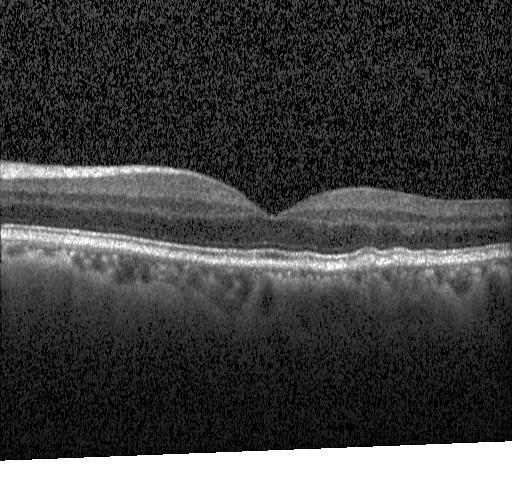 Assessment: multiple drusen.